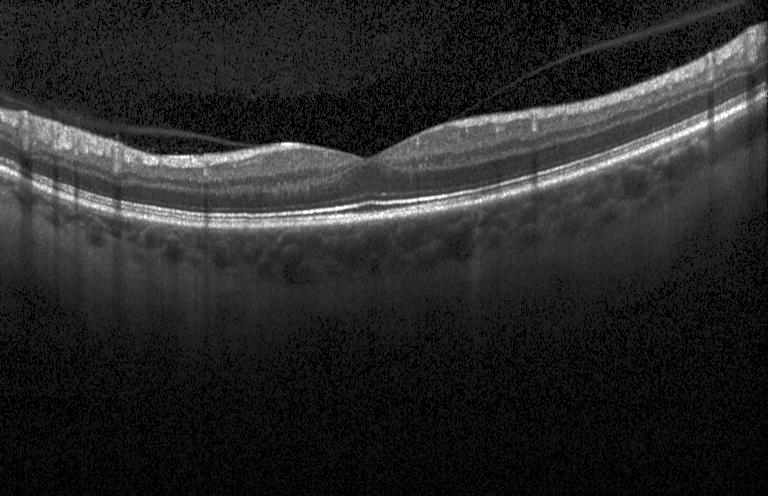

OCT line scan; spectral-domain optical coherence tomography; Heidelberg Spectralis; macular scan — Finding: no evidence of CNV, DME, or drusen.